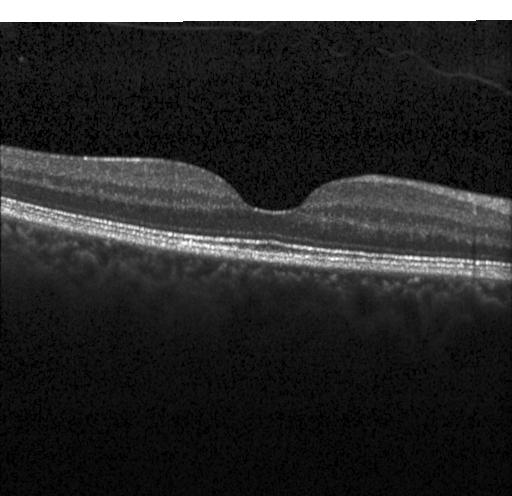 Instrument: Heidelberg Spectralis; fovea-centered; SD-OCT; retinal OCT B-scan.
Impression: no choroidal neovascularization, no diabetic macular edema, and no drusen.